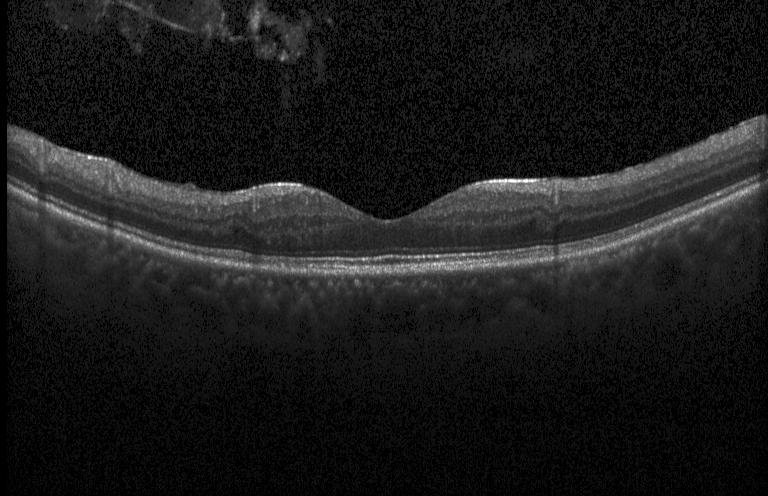
Retinal OCT cross-section showing no evidence of choroidal neovascularization, diabetic macular edema, or drusen.